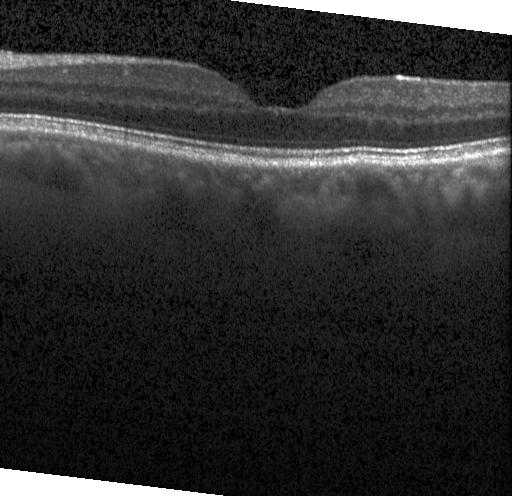

Heidelberg Spectralis, macular scan, optical coherence tomography B-scan, spectral-domain OCT. Neither choroidal neovascularization, diabetic macular edema, nor drusen.